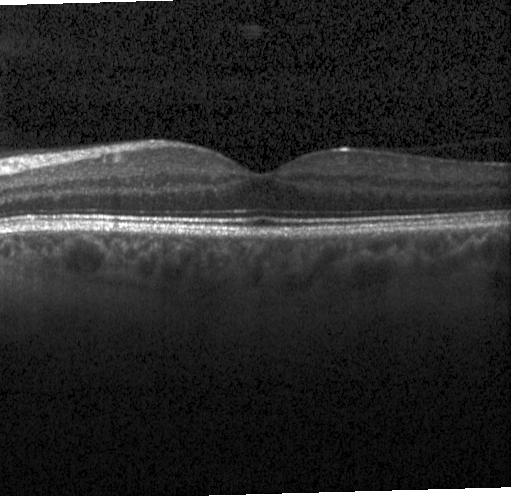

OCT finding: no evidence of choroidal neovascularization, diabetic macular edema, or drusen.